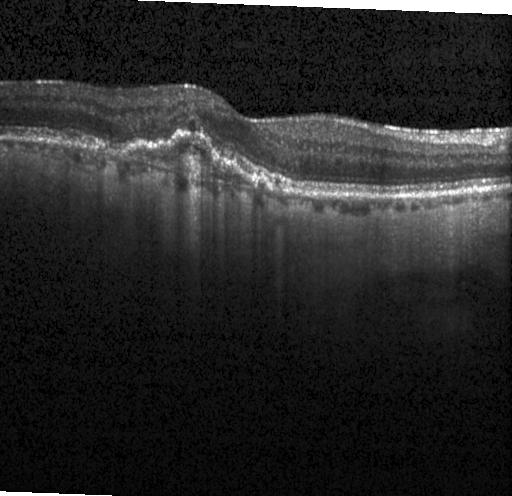
Optical coherence tomography B-scan. Instrument: Heidelberg Spectralis. Through the macula
Diagnosis: a choroidal neovascular membrane.